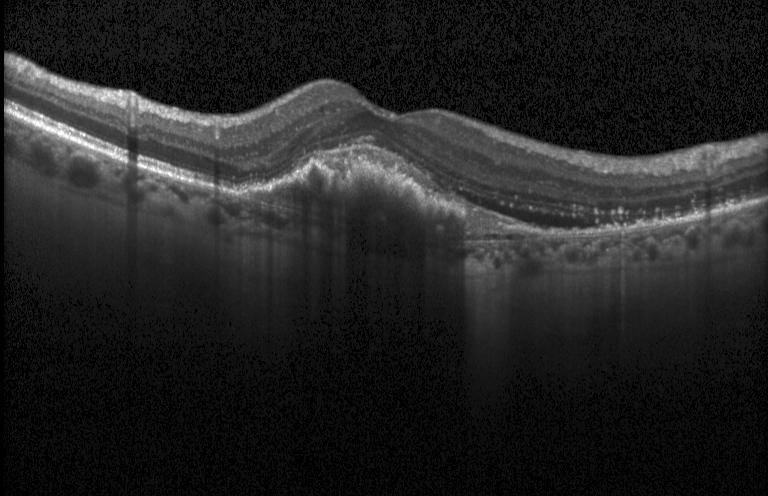 Retinal OCT B-scan. Spectral-domain OCT. Horizontal scan through the fovea. Heidelberg Spectralis OCT system.
Dx: a choroidal neovascular membrane.